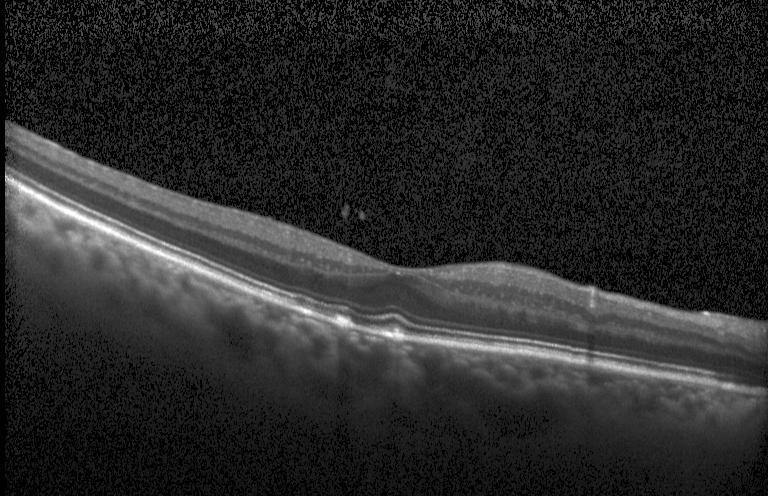

Retinal OCT B-scan, spectral-domain OCT — Finding: drusen.